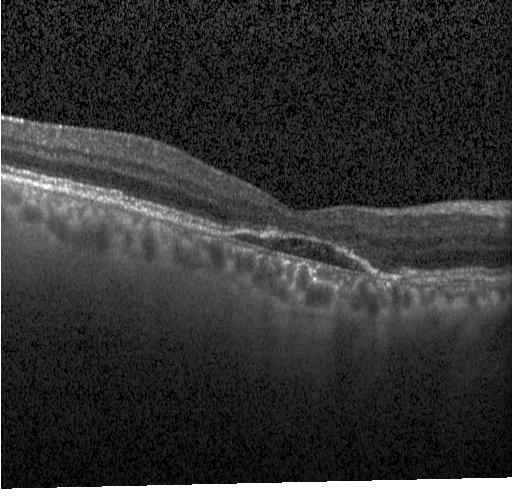 Macular OCT: choroidal neovascularization.